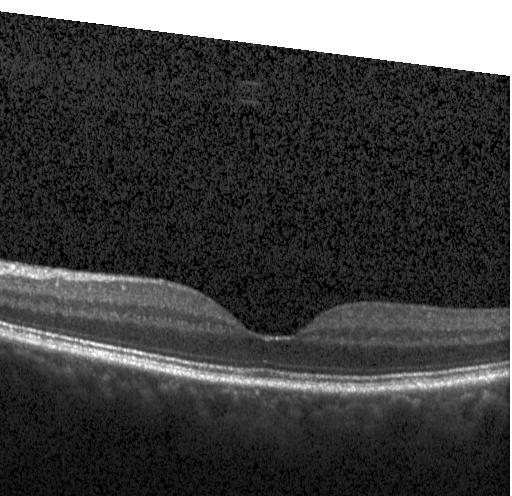
Optical coherence tomography B-scan · SD-OCT
Macular OCT: no evidence of choroidal neovascularization, diabetic macular edema, or drusen.